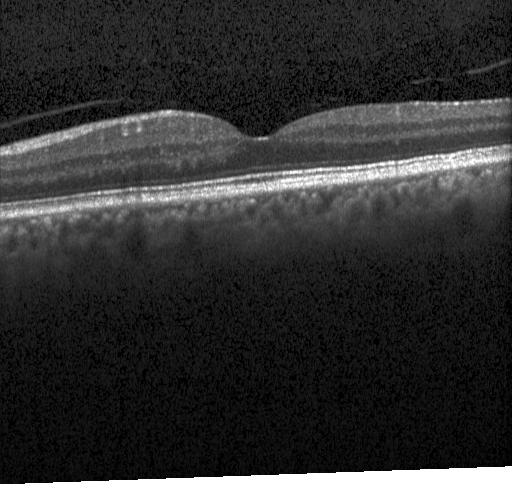 Optical coherence tomography scan. Centered on the fovea. Instrument: Heidelberg Spectralis. SD-OCT.
Diagnosis: neither CNV, DME, nor drusen.